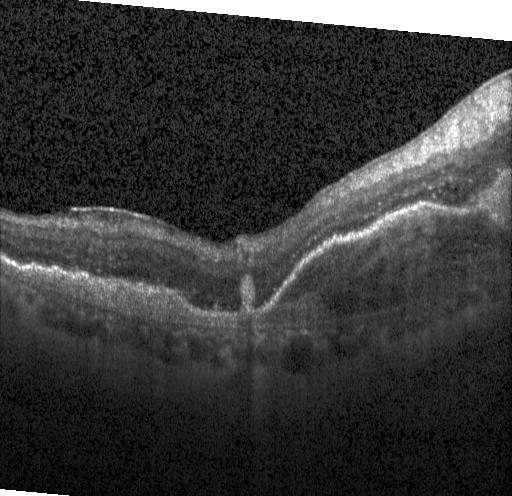 OCT line scan — OCT finding: choroidal neovascularization (CNV).